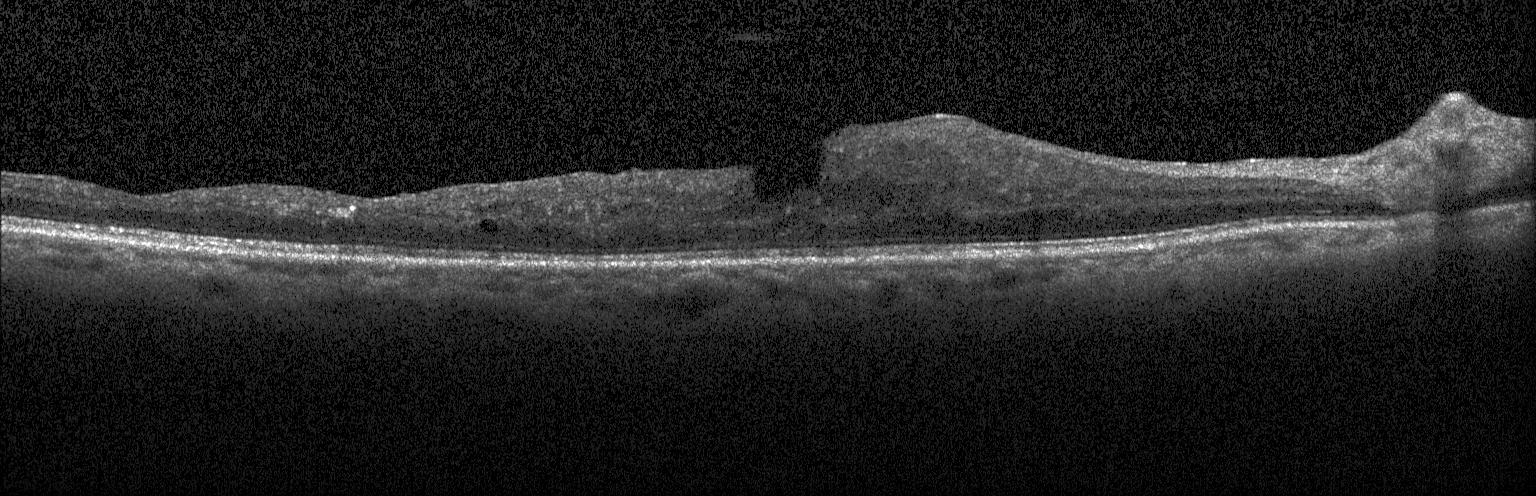

SD-OCT · OCT line scan. Impression: diabetic macular edema.